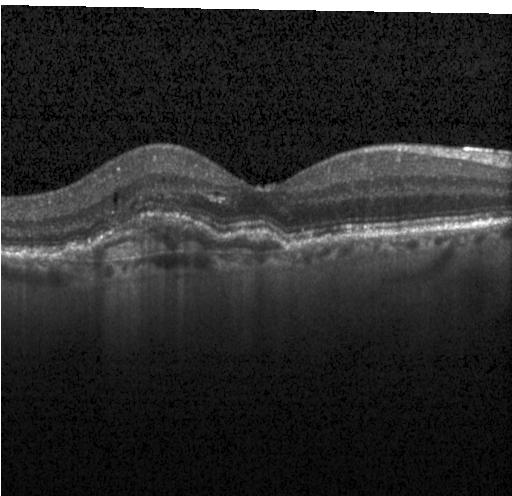 Dx: a choroidal neovascular membrane.